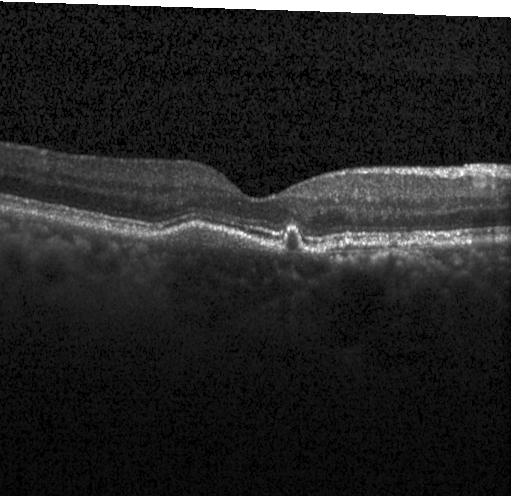
Instrument: Heidelberg Spectralis, optical coherence tomography B-scan — Impression: multiple drusen.